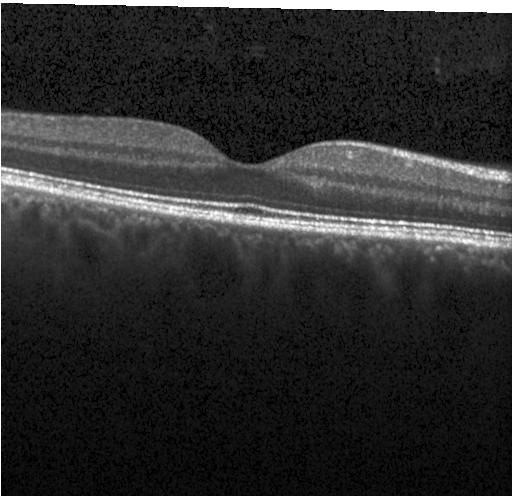 The scan shows no choroidal neovascularization, no diabetic macular edema, and no drusen.